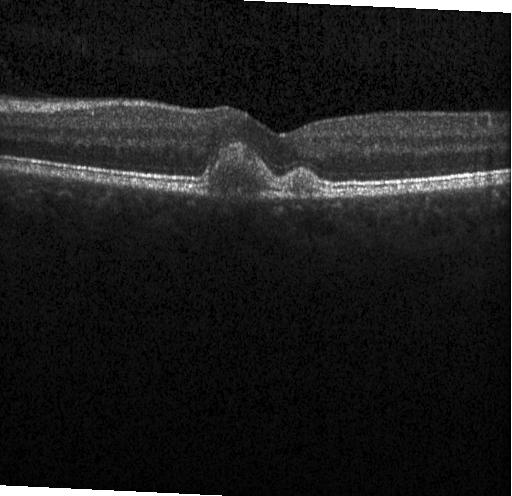

Fovea-centered · OCT line scan. Finding: drusen.